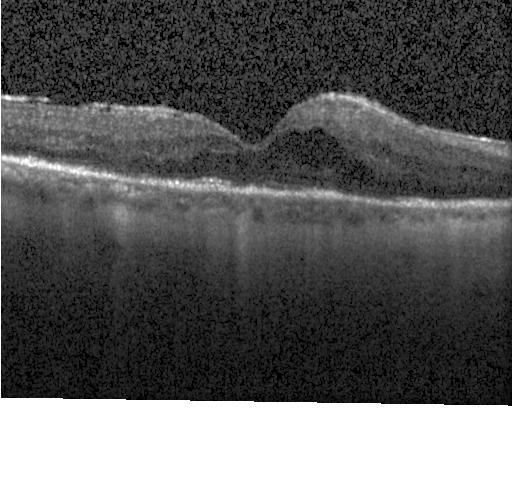
Retinal OCT B-scan; acquired on a Heidelberg Spectralis.
Impression: DME.